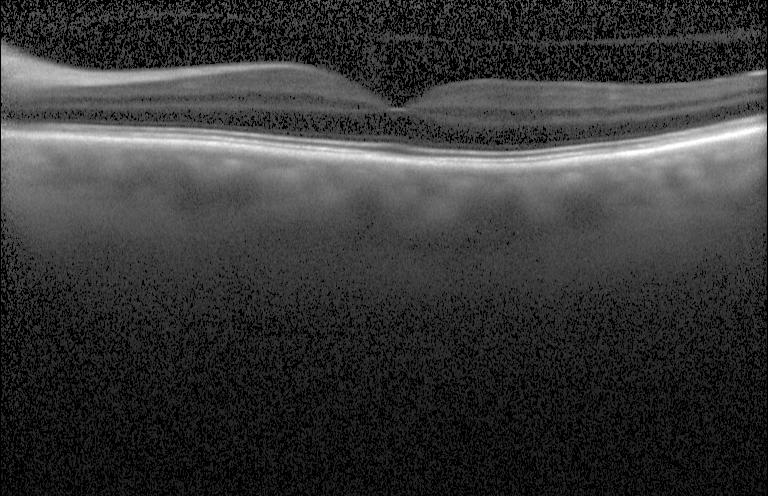 Centered on the fovea, spectral-domain OCT, instrument: Heidelberg Spectralis, OCT line scan.
Diagnosis: neither CNV, DME, nor drusen.